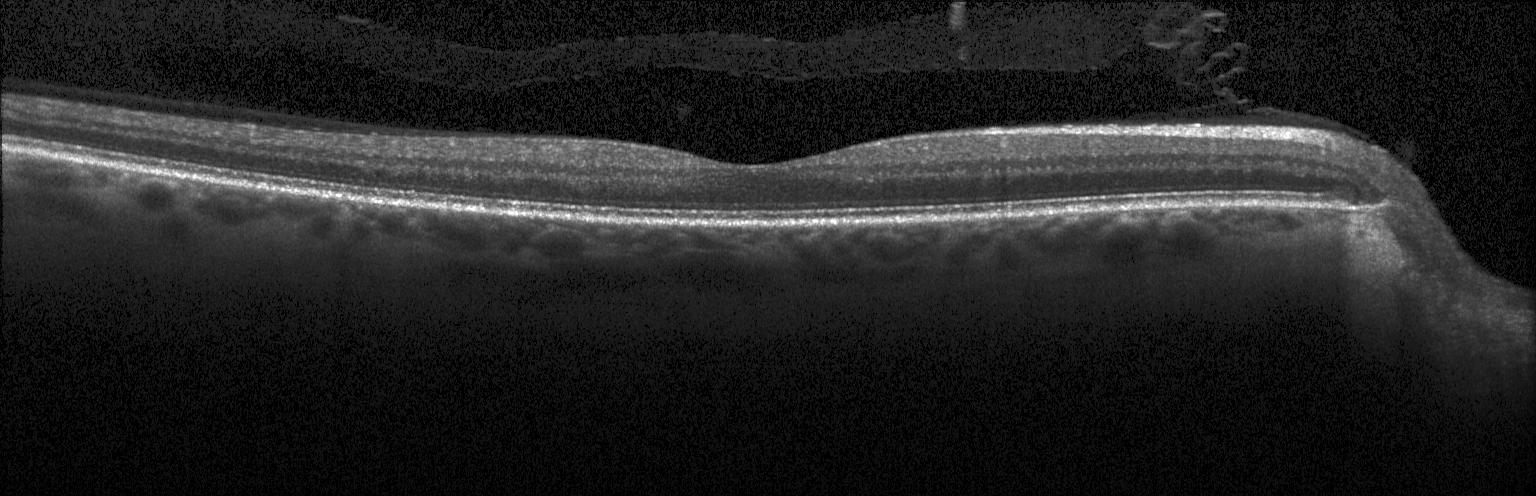

SD-OCT · optical coherence tomography scan · fovea-centered
Neither choroidal neovascularization, diabetic macular edema, nor drusen.